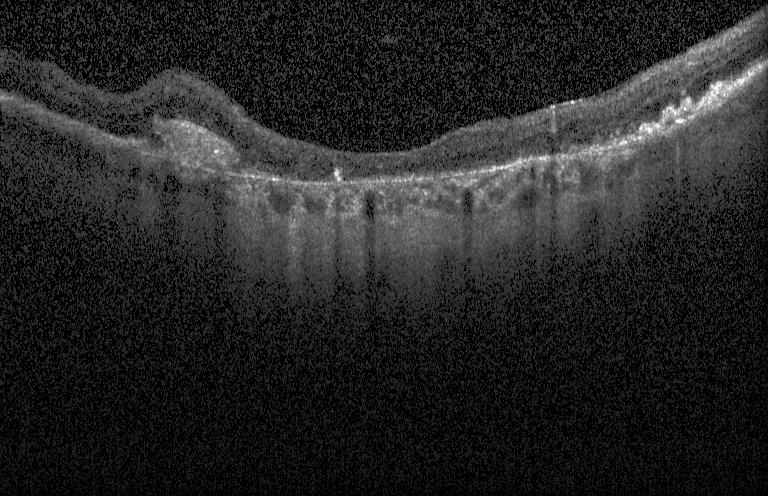 OCT B-scan.
This B-scan demonstrates choroidal neovascularization (CNV).